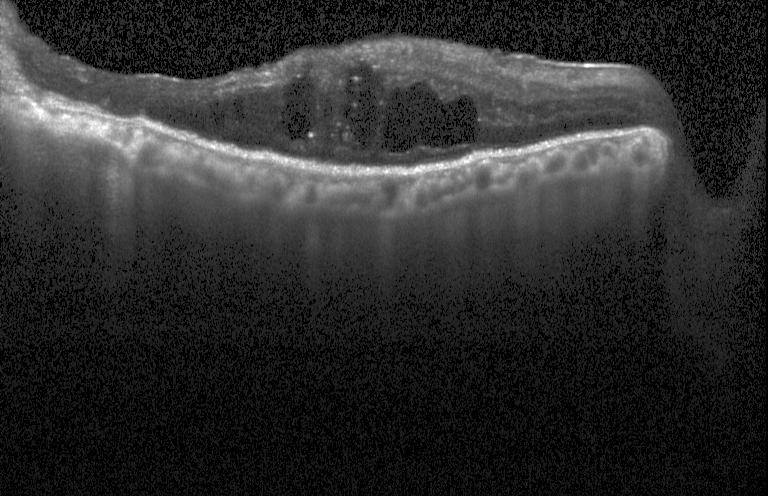 Centered on the fovea, retinal OCT cross-section, instrument: Heidelberg Spectralis, spectral-domain optical coherence tomography. Macular OCT: DME.